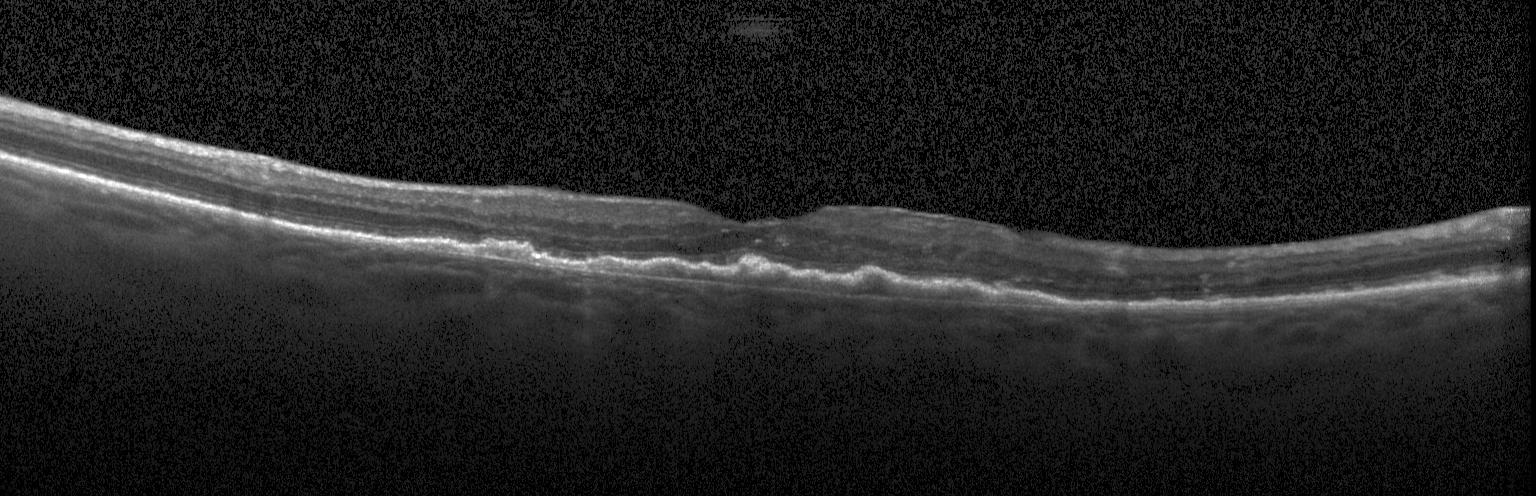
Finding: choroidal neovascularization (CNV).